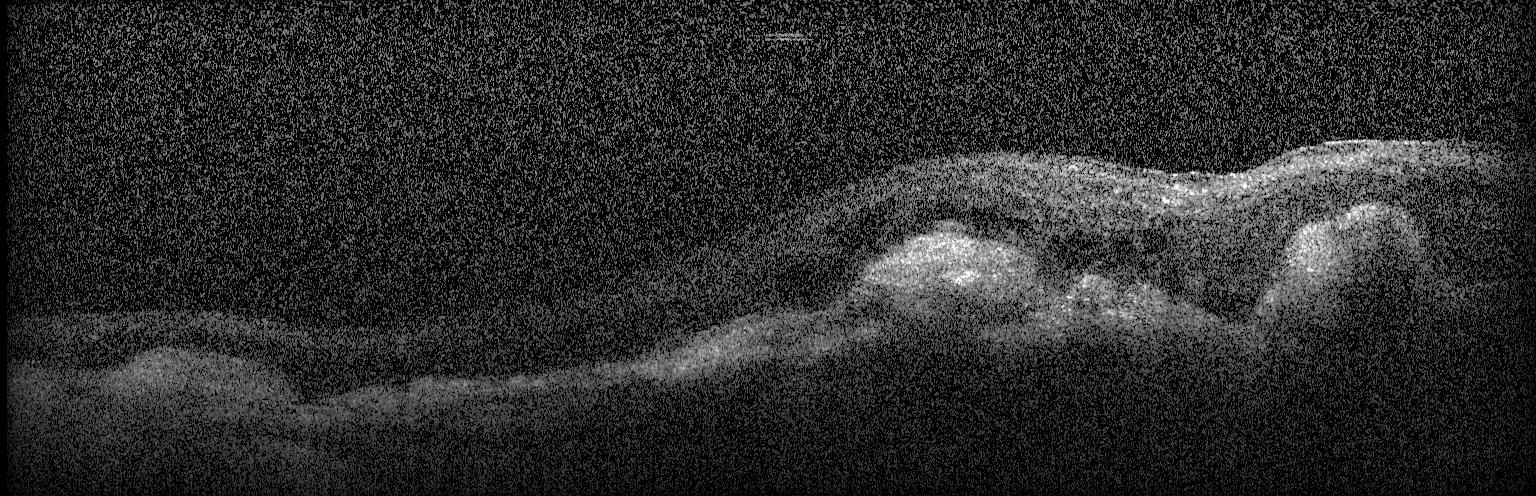
Macular OCT: choroidal neovascularization (CNV).